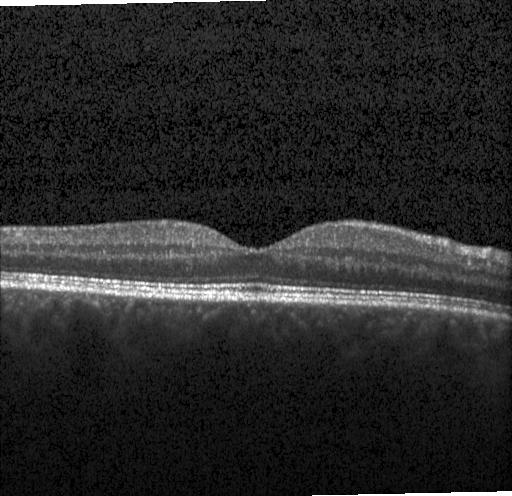 OCT line scan. Diagnosis: no choroidal neovascularization, no diabetic macular edema, and no drusen.